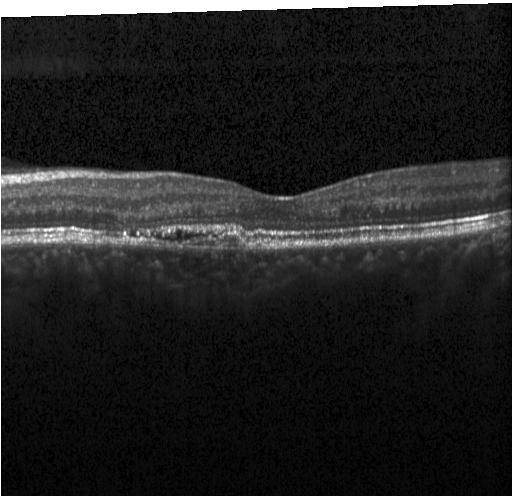

Finding: choroidal neovascularization (CNV).